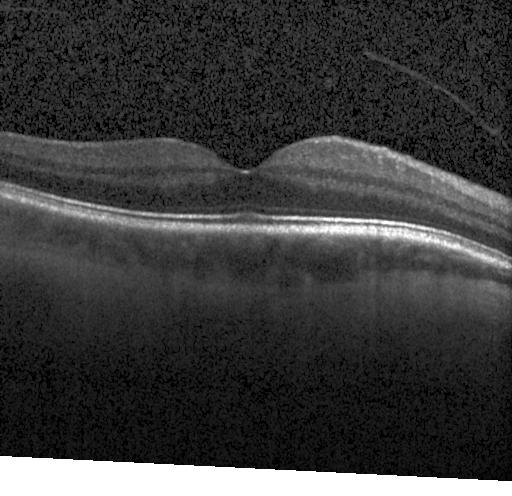

SD-OCT. Heidelberg Spectralis OCT system. Retinal OCT cross-section. Through the macula — This B-scan demonstrates no evidence of CNV, DME, or drusen.